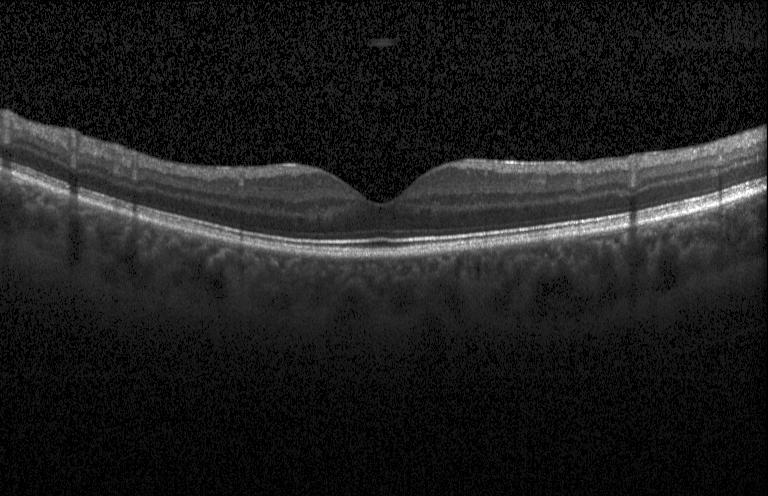
Diagnosis: neither choroidal neovascularization, diabetic macular edema, nor drusen.